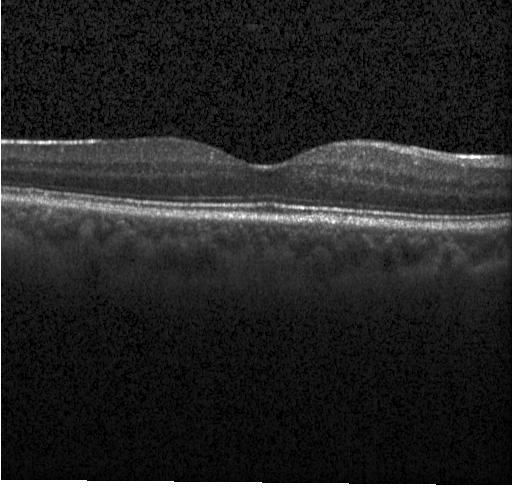

Retinal OCT B-scan. Spectral-domain optical coherence tomography.
No choroidal neovascularization, no diabetic macular edema, and no drusen.